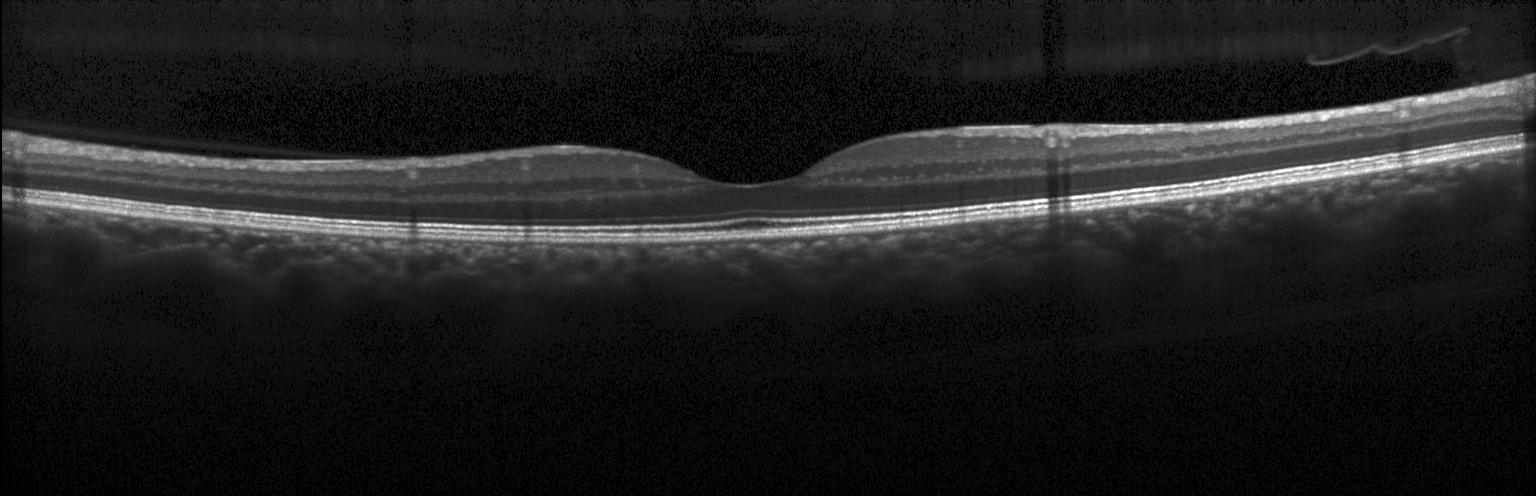 Heidelberg Spectralis OCT system. SD-OCT. Through the macula. OCT B-scan.
OCT finding: no choroidal neovascularization, diabetic macular edema, or drusen.